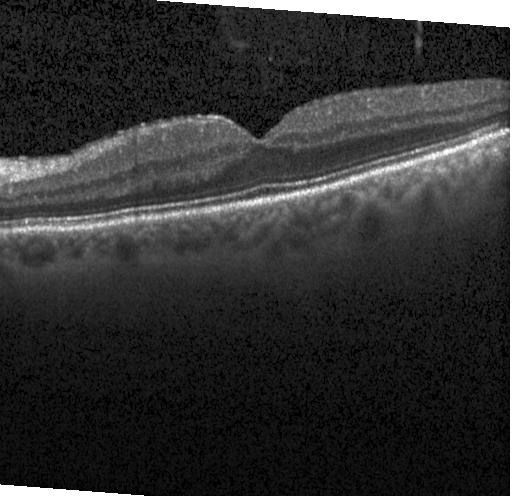 Heidelberg Spectralis. Retinal OCT cross-section
Assessment: neither choroidal neovascularization, diabetic macular edema, nor drusen.